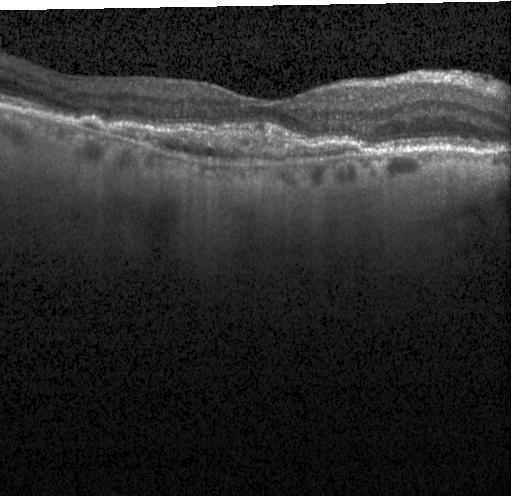 Acquired on a Heidelberg Spectralis. Retinal OCT B-scan. Spectral-domain OCT. Fovea-centered — This B-scan demonstrates a choroidal neovascular membrane.